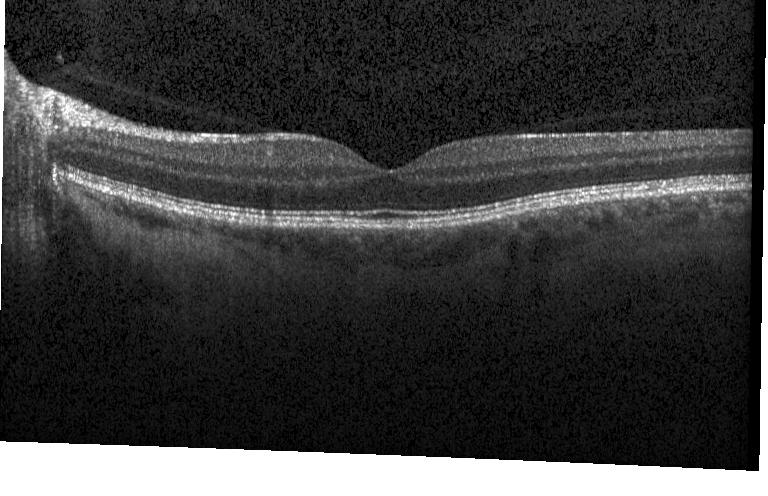 Centered on the fovea. Heidelberg Spectralis OCT system. Spectral-domain optical coherence tomography. Optical coherence tomography B-scan — Macular OCT: neither CNV, DME, nor drusen.